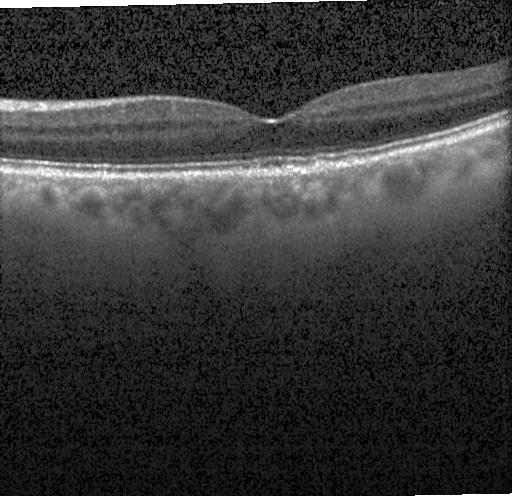

OCT line scan, spectral-domain optical coherence tomography, fovea-centered. The scan shows drusen.